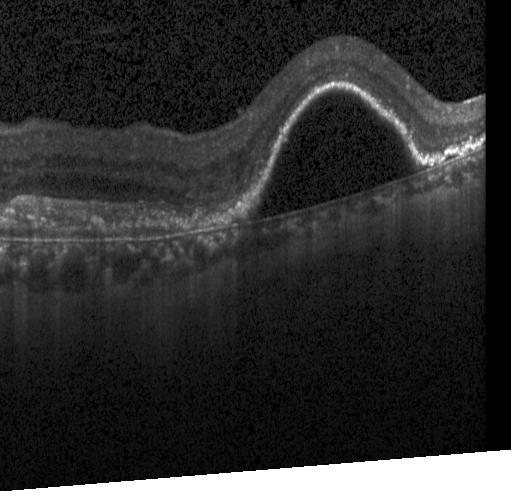 Centered on the fovea. Acquired on a Heidelberg Spectralis. Optical coherence tomography B-scan. Spectral-domain OCT. The scan shows a choroidal neovascular membrane.